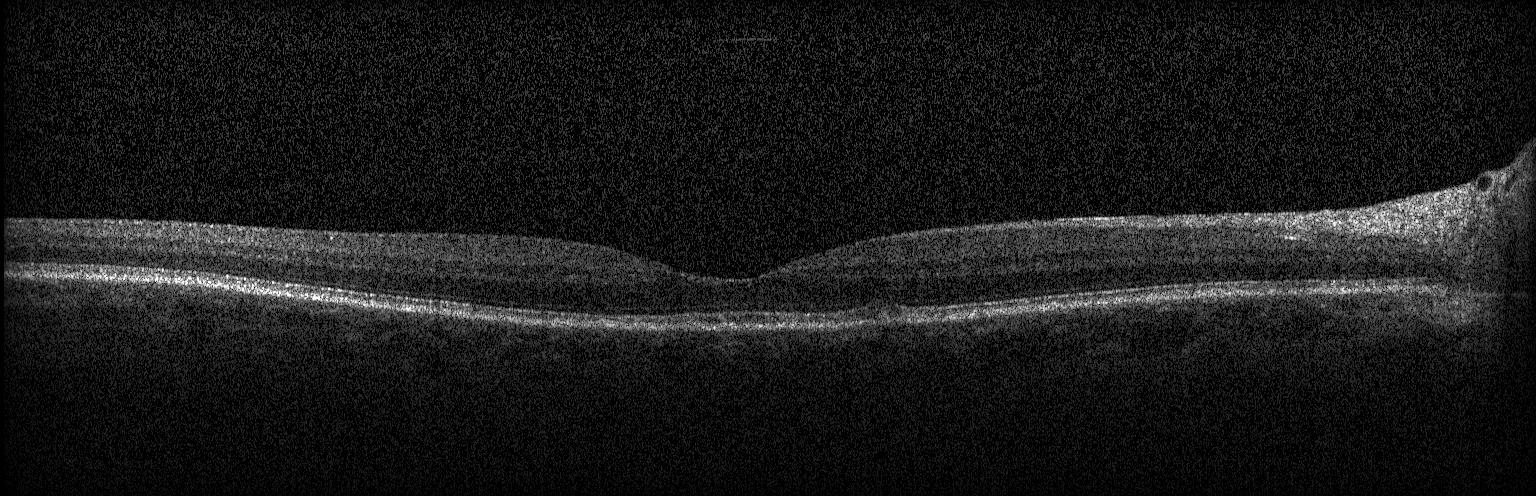 Finding: no choroidal neovascularization, diabetic macular edema, or drusen.